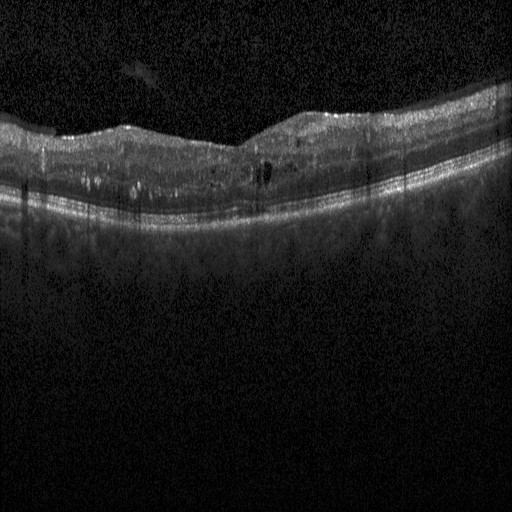 OCT line scan — The scan shows diabetic macular edema.